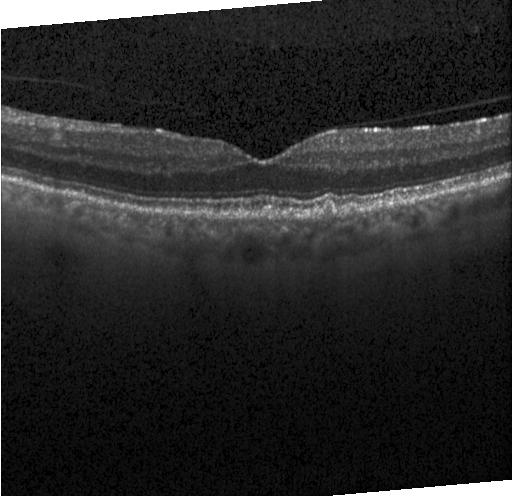
Acquired on a Heidelberg Spectralis, OCT B-scan, horizontal scan through the fovea
Diagnosis: drusen.